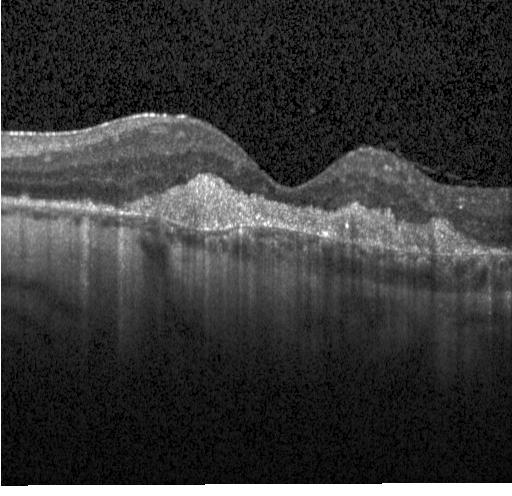

Spectral-domain OCT. OCT line scan. Assessment: a choroidal neovascular membrane.